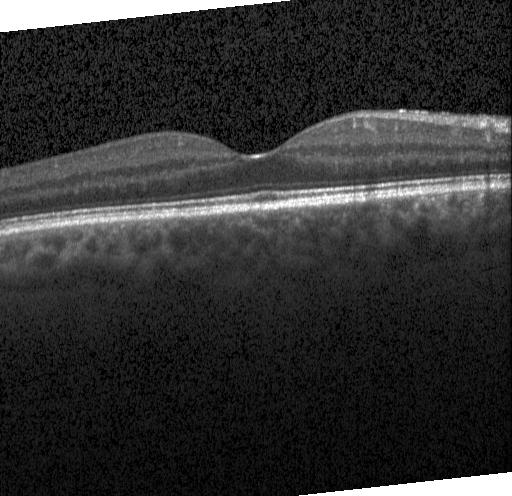
The scan shows no CNV, no DME, and no drusen.